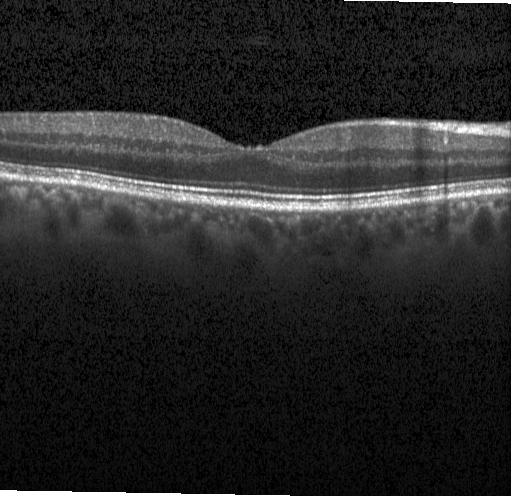

Acquired on a Heidelberg Spectralis; spectral-domain OCT; optical coherence tomography B-scan — Diagnosis: neither CNV, DME, nor drusen.